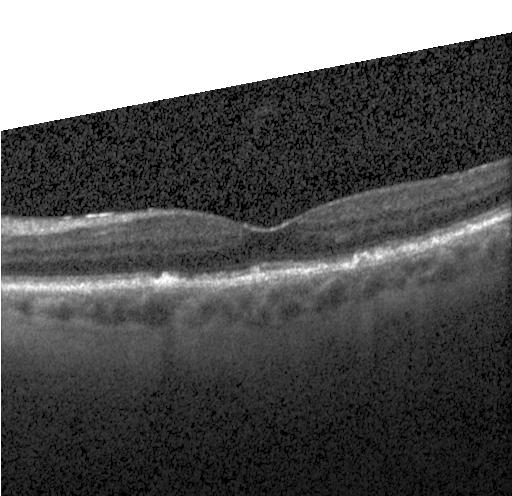

Fovea-centered, SD-OCT, OCT B-scan
Finding: drusen.